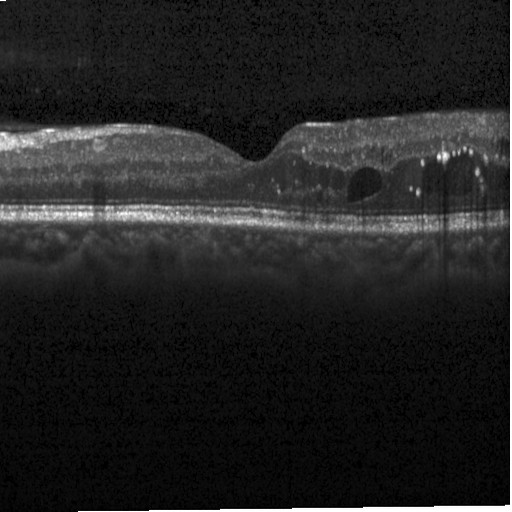
Retinal OCT B-scan, horizontal scan through the fovea, spectral-domain optical coherence tomography, Heidelberg Spectralis — Impression: diabetic macular edema.